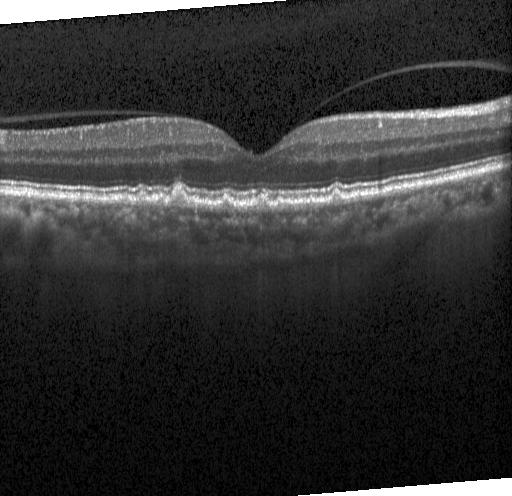 The scan shows sub-RPE drusenoid deposits.